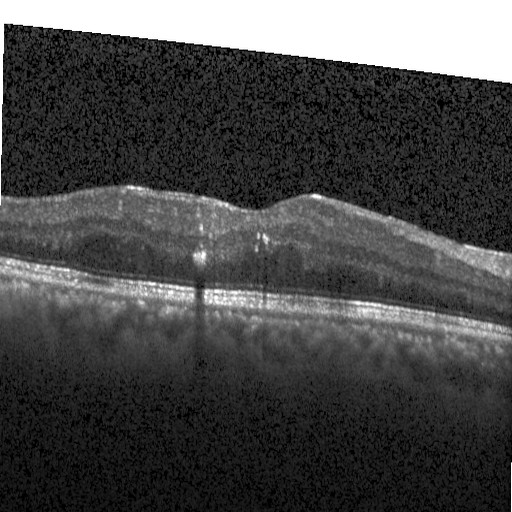

Dx: DME.